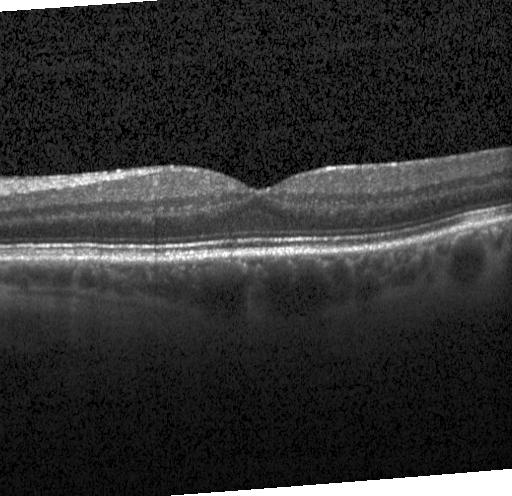
Finding: no evidence of CNV, DME, or drusen.